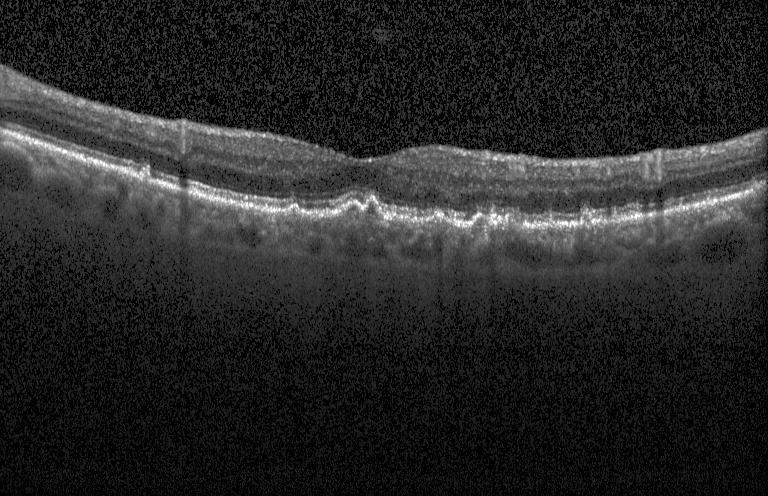
Impression: sub-RPE drusenoid deposits.